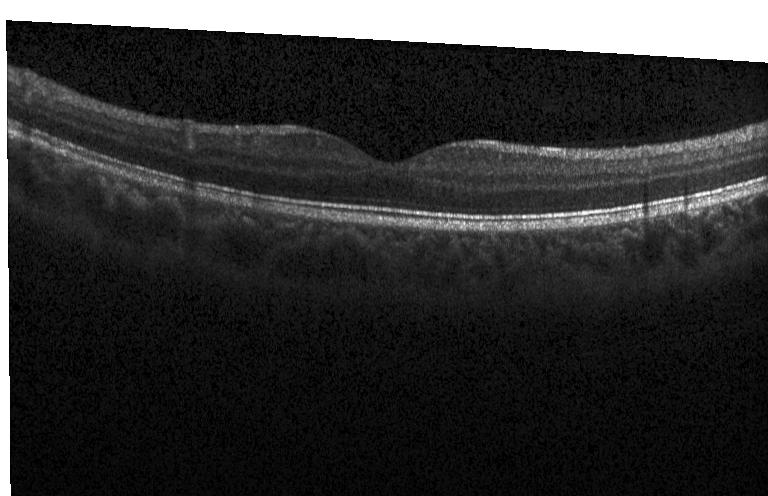 Diagnosis: no CNV, DME, or drusen.